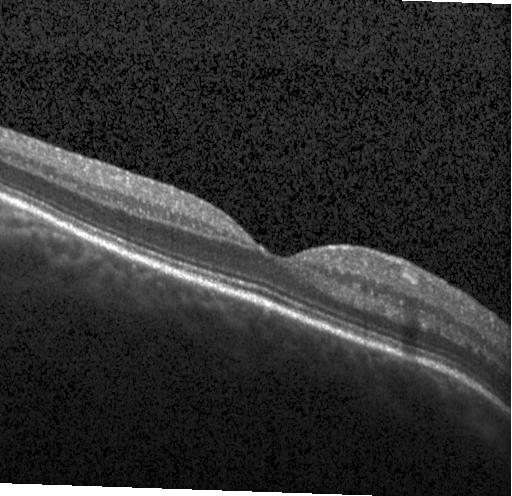

Spectral-domain optical coherence tomography. OCT B-scan
Assessment: no choroidal neovascularization, diabetic macular edema, or drusen.